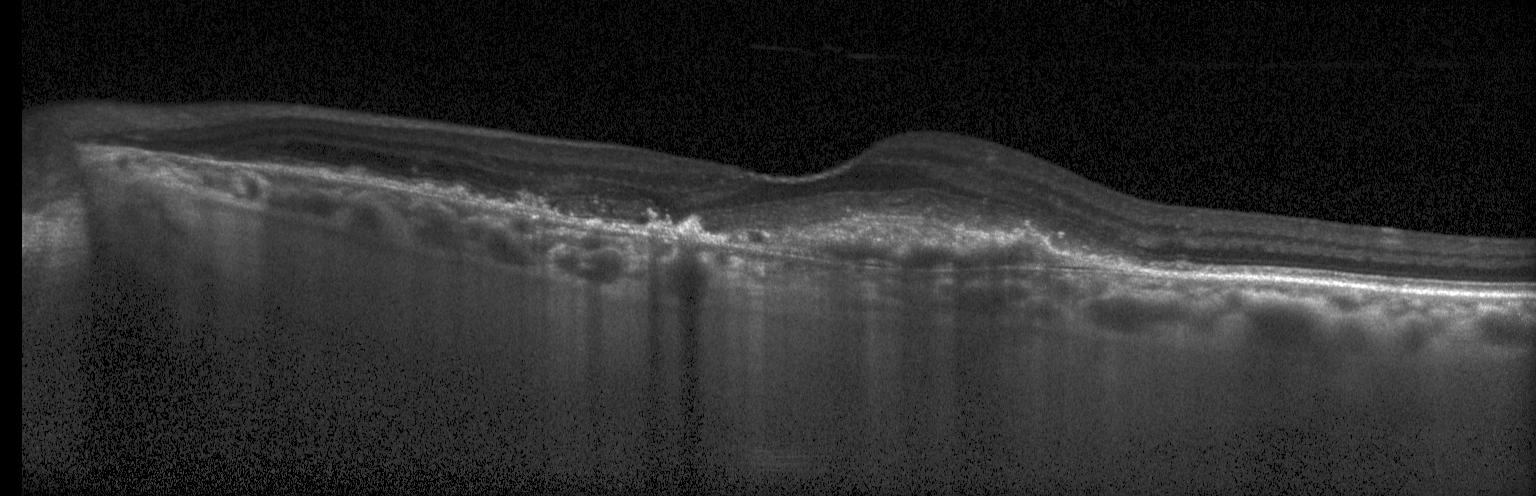 Dx: a choroidal neovascular membrane.